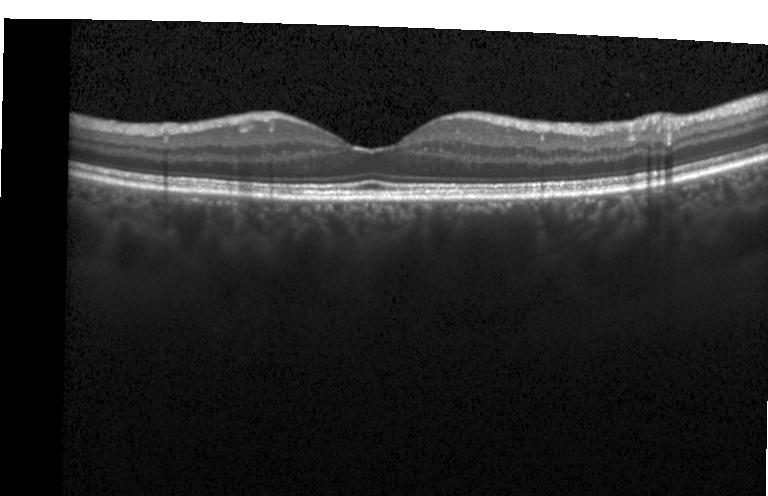
Optical coherence tomography B-scan. Macular scan. Spectral-domain OCT
Macular OCT: no CNV, no DME, and no drusen.